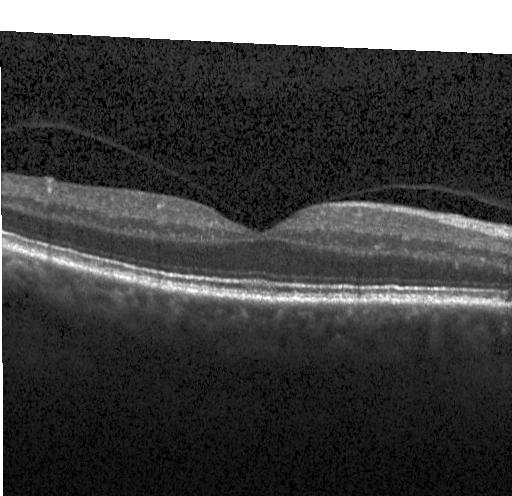
Retinal OCT cross-section
Impression: no choroidal neovascularization, no diabetic macular edema, and no drusen.